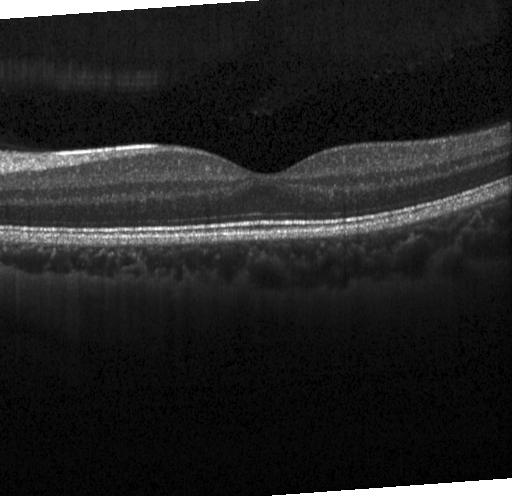

OCT finding: no evidence of choroidal neovascularization, diabetic macular edema, or drusen.